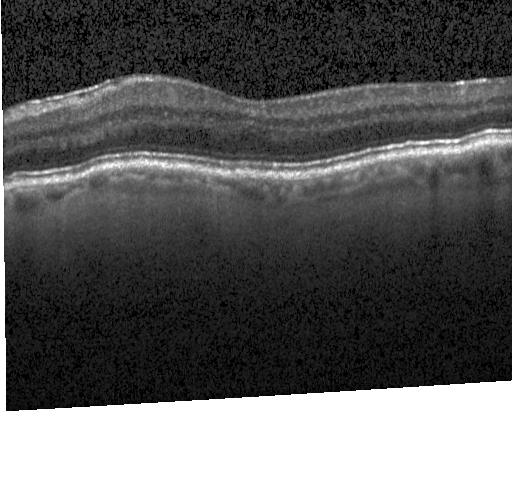
No choroidal neovascularization, no diabetic macular edema, and no drusen.